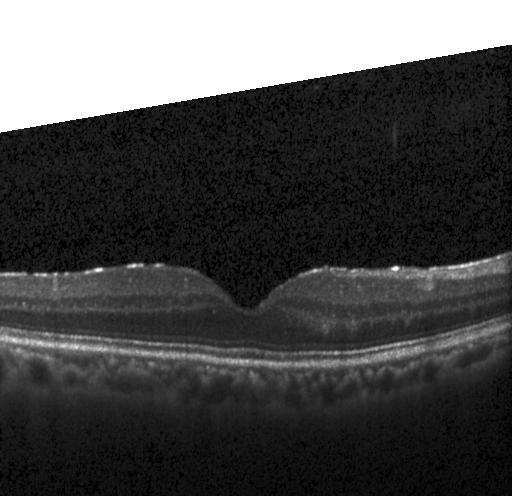

Macular OCT: no choroidal neovascularization, diabetic macular edema, or drusen.